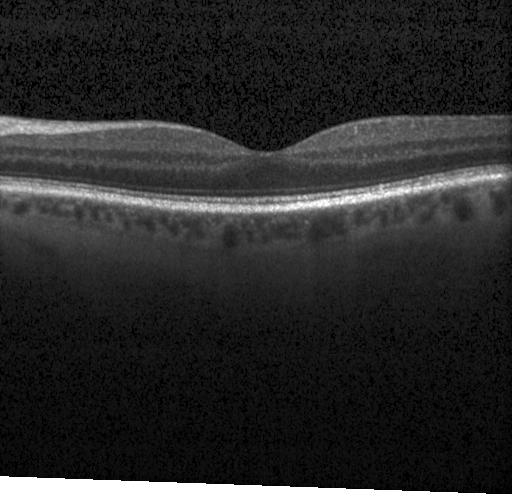

Optical coherence tomography B-scan — Dx: no evidence of choroidal neovascularization, diabetic macular edema, or drusen.